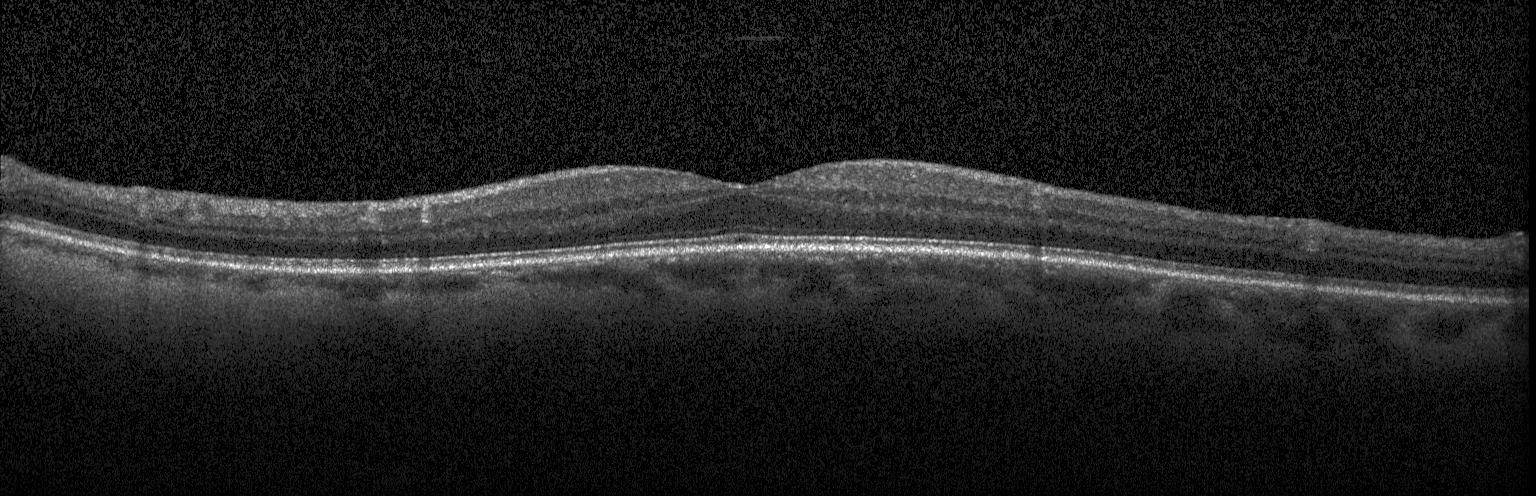

Assessment: no choroidal neovascularization, no diabetic macular edema, and no drusen.